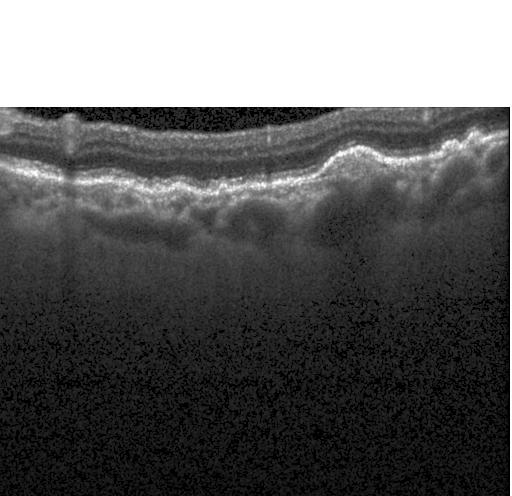
Impression: sub-RPE drusenoid deposits.